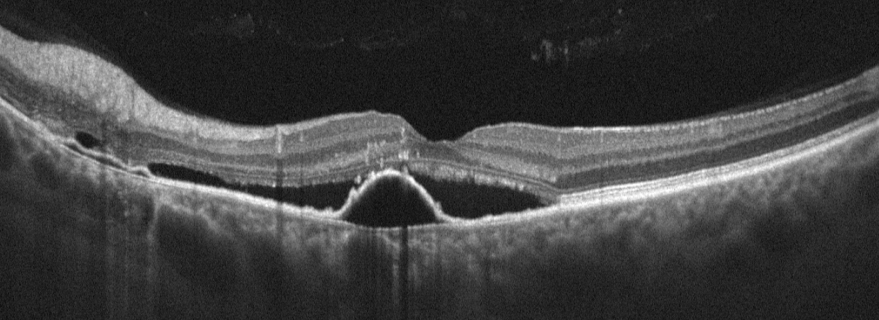

Optical coherence tomography scan; Optovue Avanti RTVue XR — Impression: AMD.